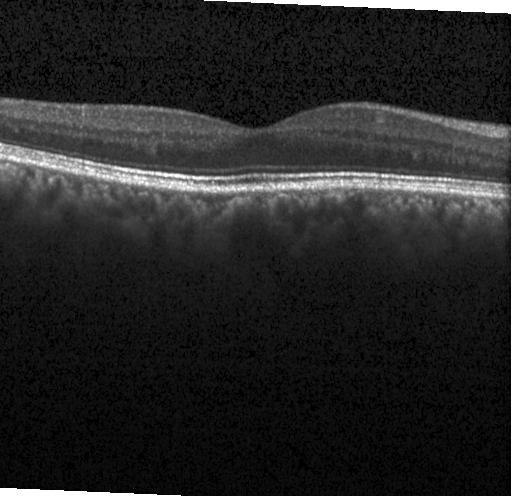
Retinal OCT B-scan — Diagnosis: no choroidal neovascularization, no diabetic macular edema, and no drusen.